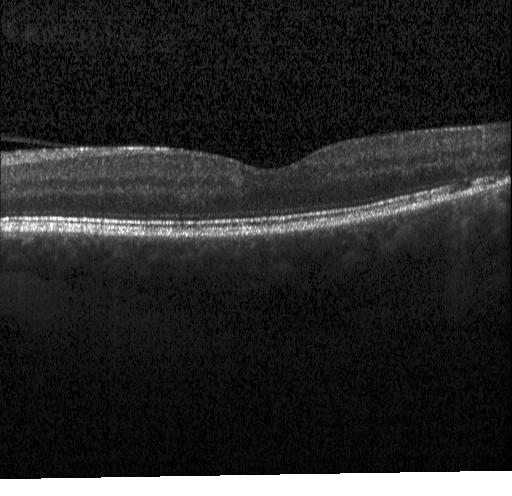 OCT line scan, through the macula
The scan shows neither choroidal neovascularization, diabetic macular edema, nor drusen.